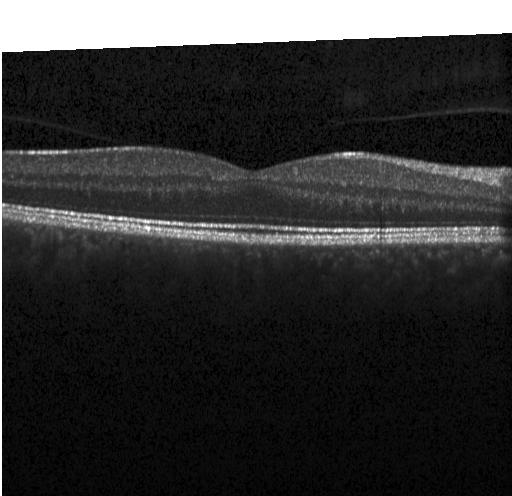

Macular OCT: no CNV, no DME, and no drusen.